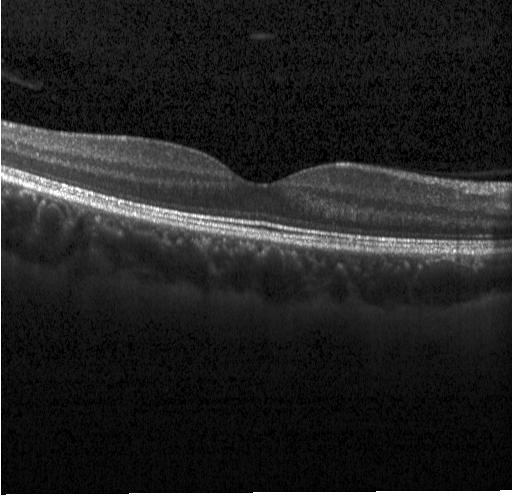

Retinal OCT cross-section showing no choroidal neovascularization, no diabetic macular edema, and no drusen.